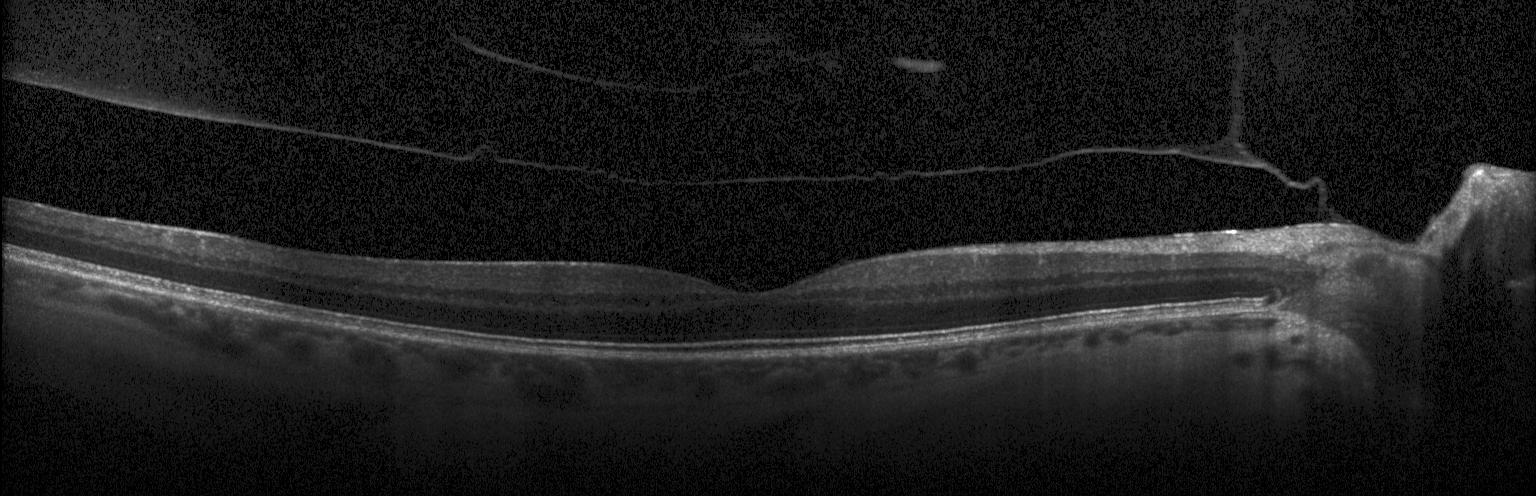 Macular OCT: no choroidal neovascularization, no diabetic macular edema, and no drusen.